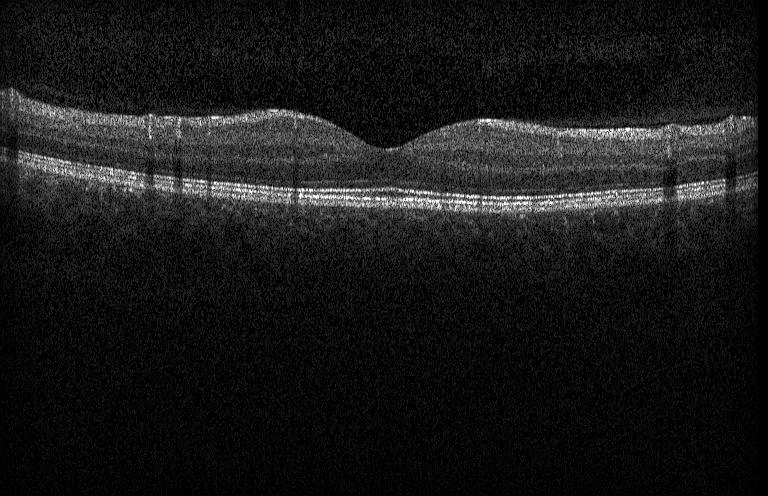
Heidelberg Spectralis OCT system, centered on the fovea, OCT B-scan — Impression: neither CNV, DME, nor drusen.